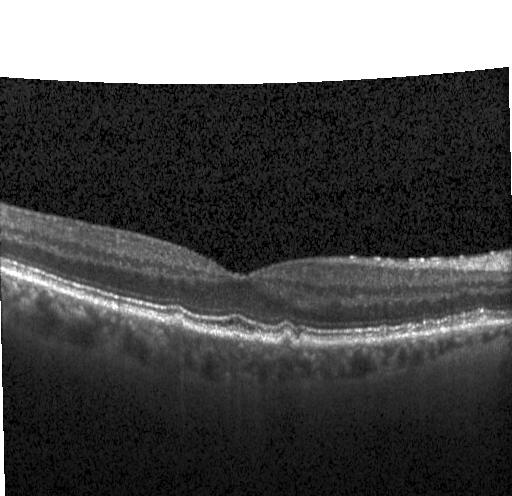 Heidelberg Spectralis; spectral-domain optical coherence tomography; optical coherence tomography B-scan
Finding: drusen.